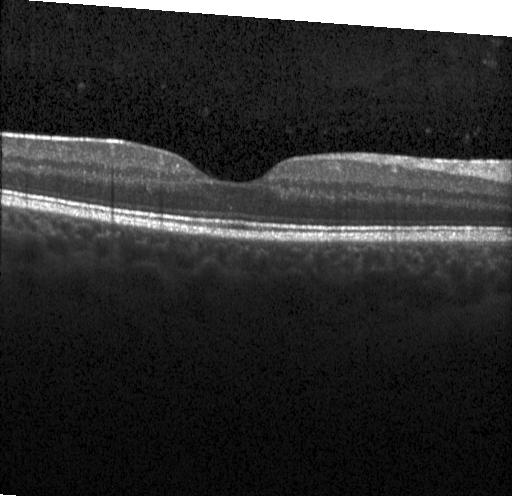

Optical coherence tomography scan; instrument: Heidelberg Spectralis; SD-OCT; fovea-centered
Diagnosis: neither choroidal neovascularization, diabetic macular edema, nor drusen.